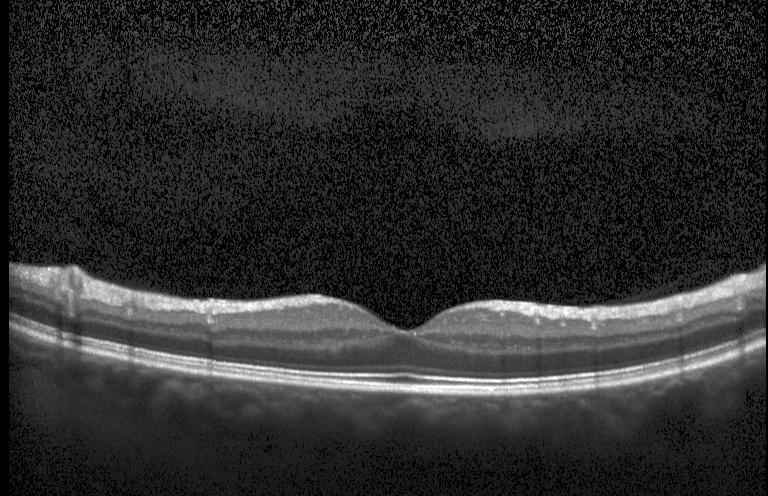
Heidelberg Spectralis · retinal OCT cross-section — This B-scan demonstrates neither choroidal neovascularization, diabetic macular edema, nor drusen.